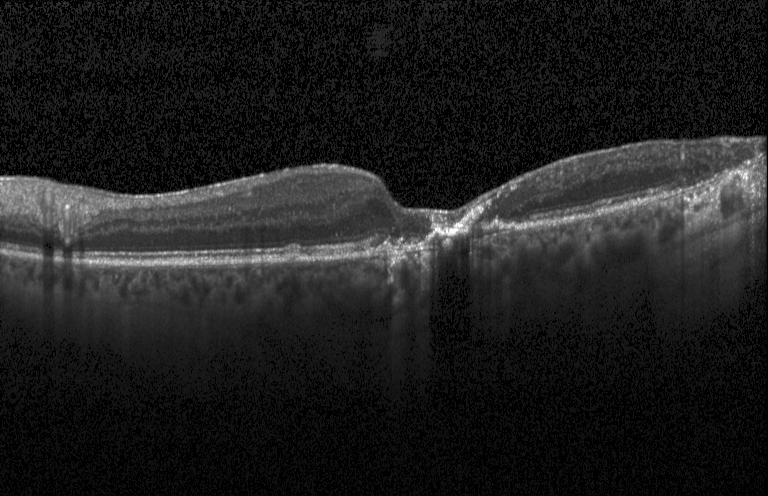

Choroidal neovascularization.